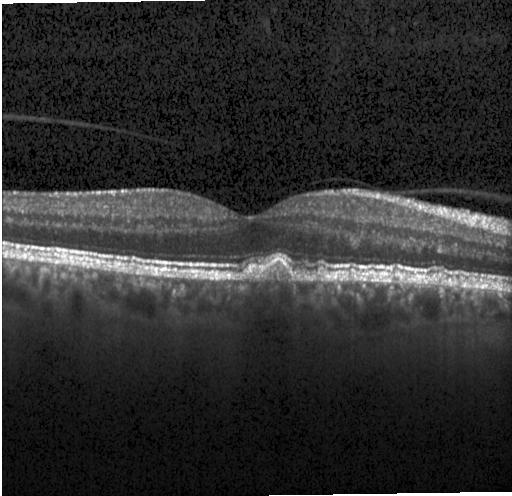 Spectral-domain optical coherence tomography; retinal OCT cross-section — Multiple drusen.